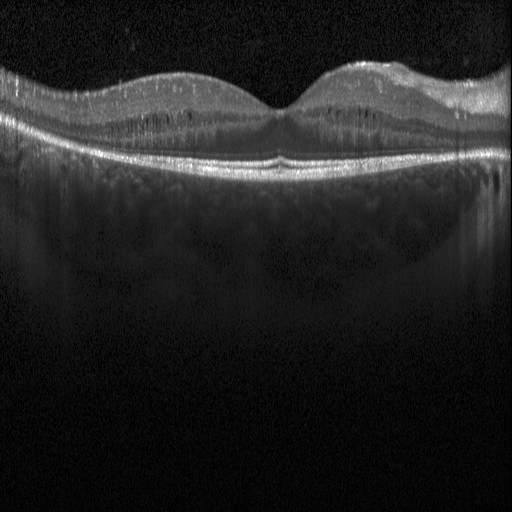 Spectral-domain OCT, optical coherence tomography scan
Diagnosis: DME.